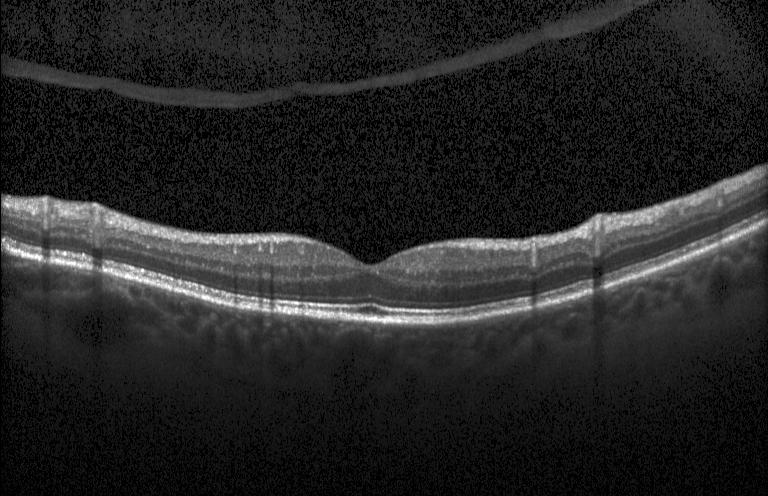
Fovea-centered; OCT line scan; spectral-domain optical coherence tomography; instrument: Heidelberg Spectralis — Finding: neither CNV, DME, nor drusen.